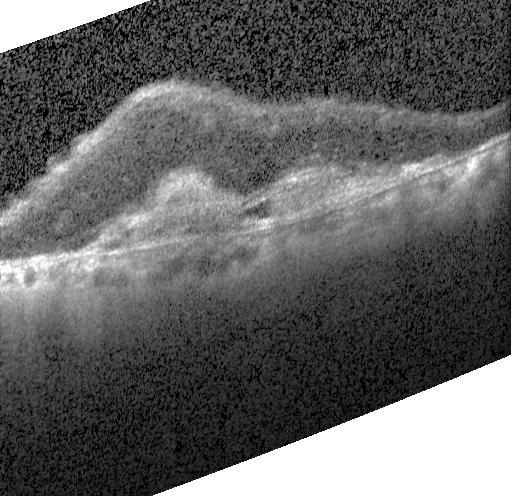

Retinal OCT B-scan, instrument: Heidelberg Spectralis — Impression: a choroidal neovascular membrane.